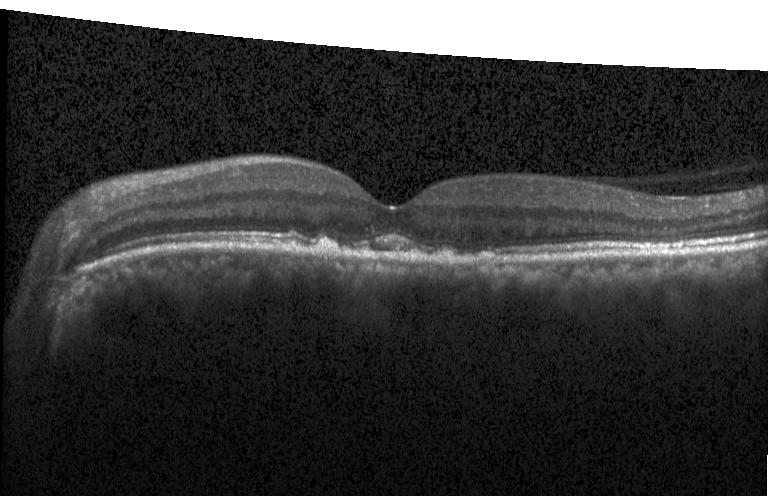
SD-OCT · OCT line scan · acquired on a Heidelberg Spectralis. Dx: choroidal neovascularization (CNV).